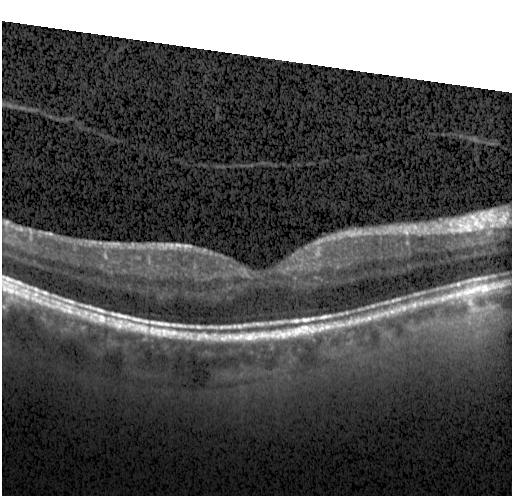

Finding: no evidence of choroidal neovascularization, diabetic macular edema, or drusen.